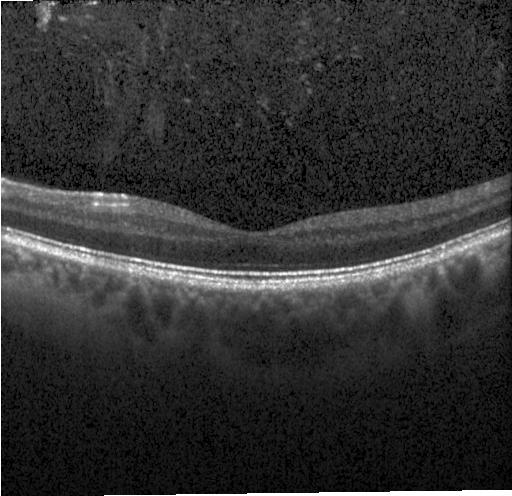

Dx: neither choroidal neovascularization, diabetic macular edema, nor drusen.